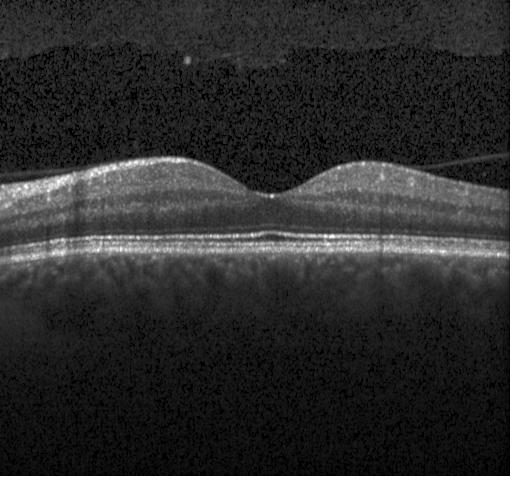 Macular OCT: no CNV, no DME, and no drusen.